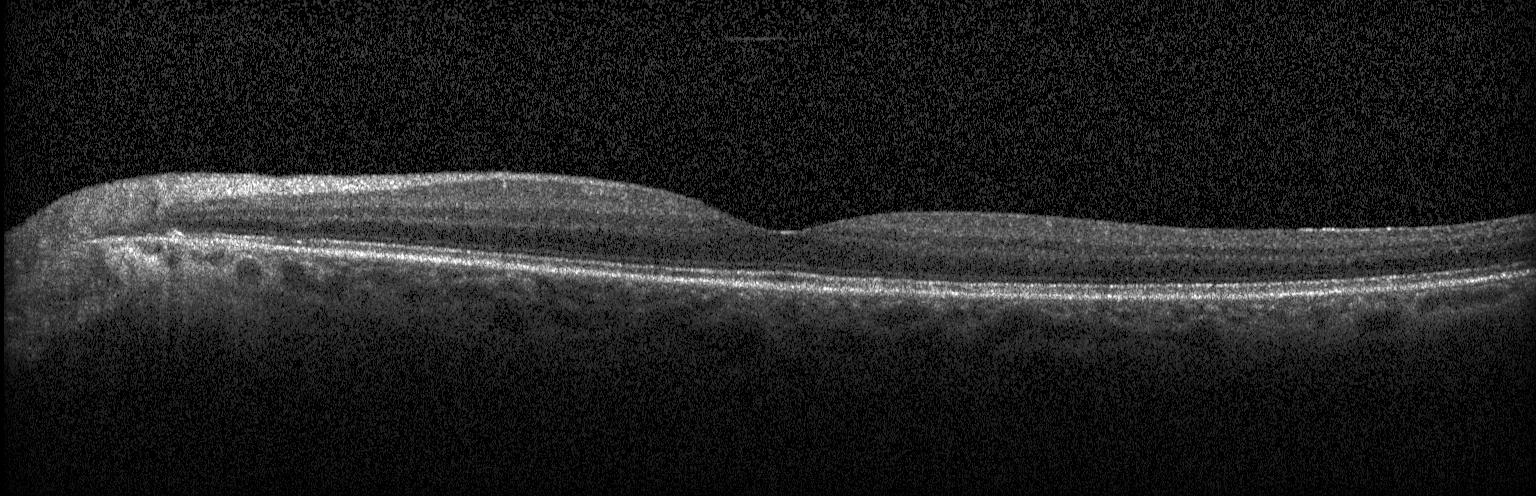

Through the macula. OCT B-scan — This B-scan demonstrates neither choroidal neovascularization, diabetic macular edema, nor drusen.